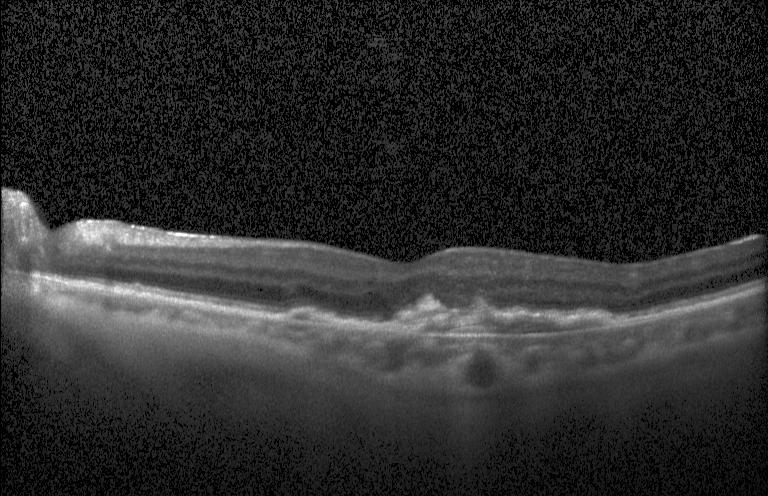
OCT line scan. Diagnosis: a choroidal neovascular membrane.